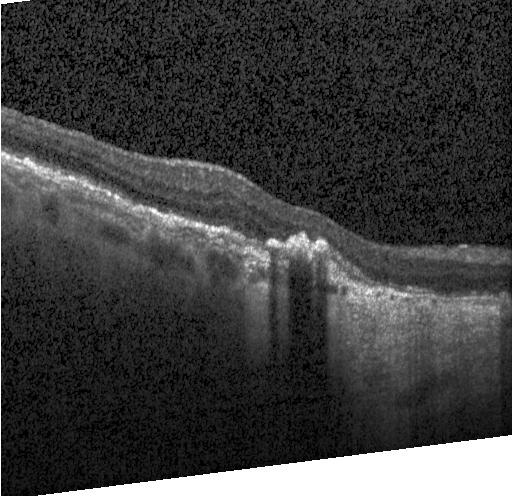
Retinal OCT cross-section · SD-OCT · Heidelberg Spectralis OCT system — The scan shows a choroidal neovascular membrane.